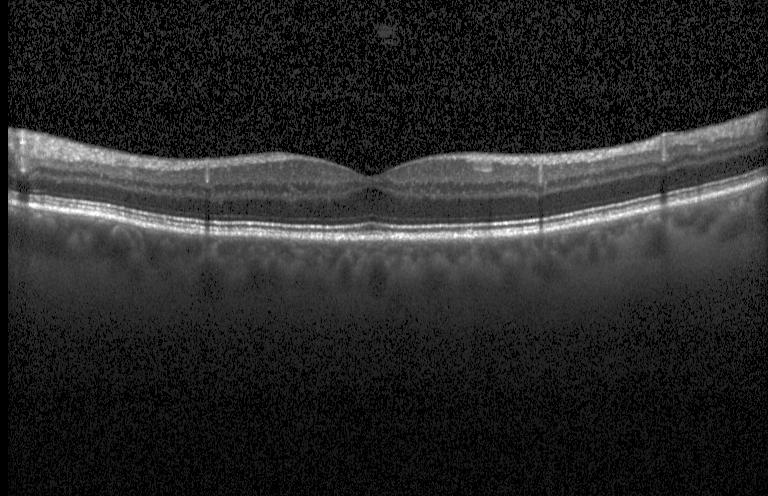

OCT B-scan.
Assessment: neither choroidal neovascularization, diabetic macular edema, nor drusen.